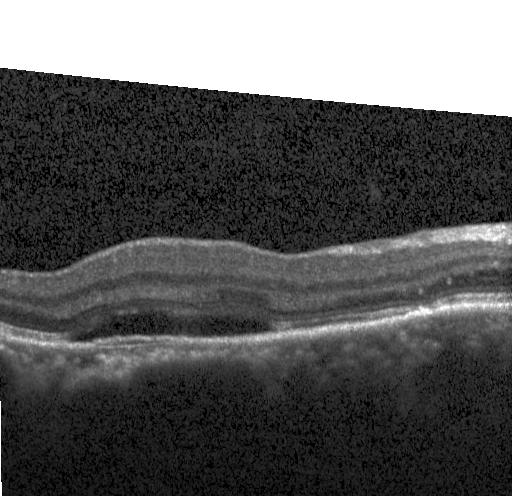 OCT B-scan · through the macula. Choroidal neovascularization.